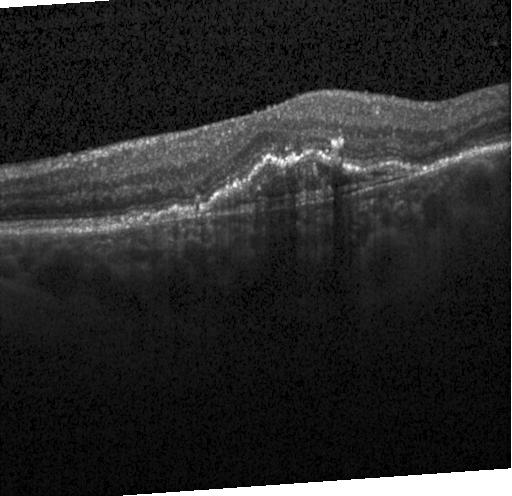 Retinal OCT B-scan
Diagnosis: a choroidal neovascular membrane.